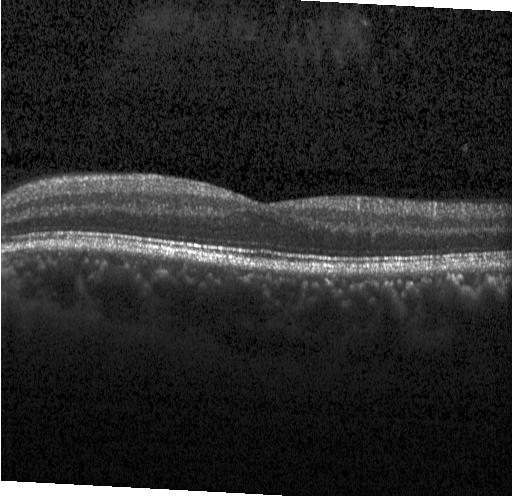
OCT finding: no CNV, DME, or drusen.